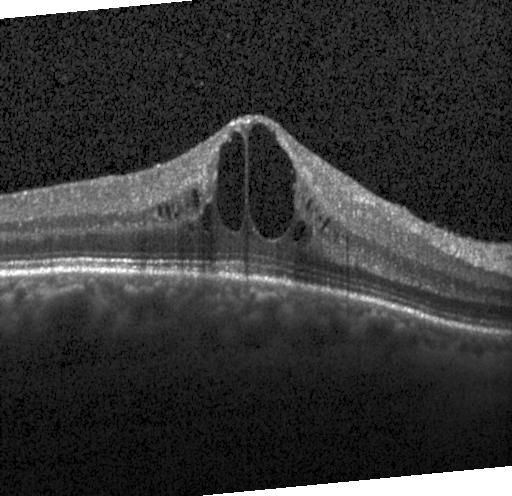 The scan shows DME.